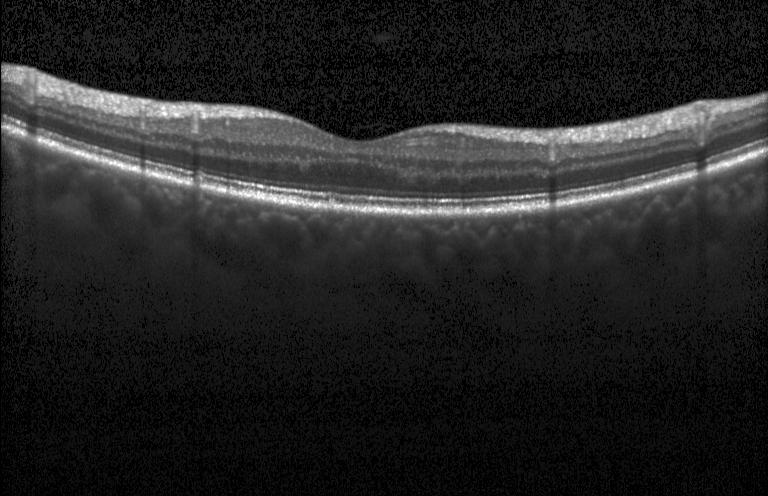
Finding: no choroidal neovascularization, no diabetic macular edema, and no drusen.